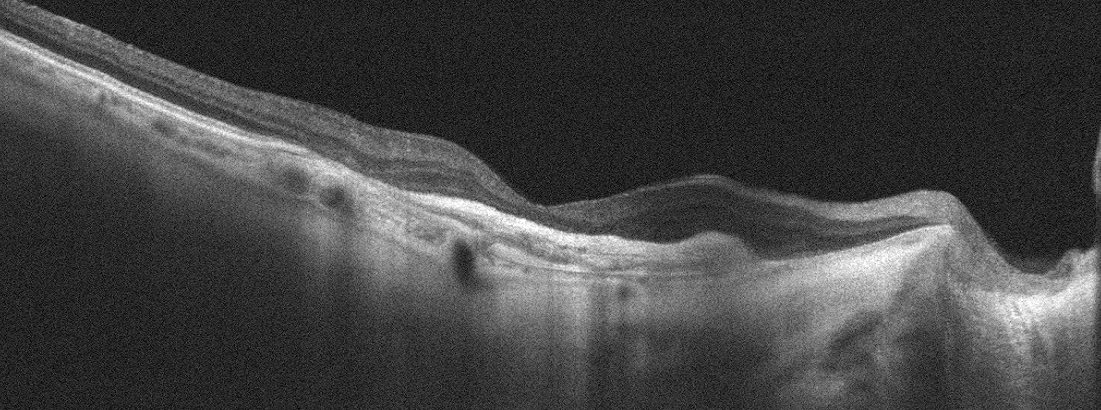
Optical coherence tomography scan.
Impression: age-related macular degeneration.